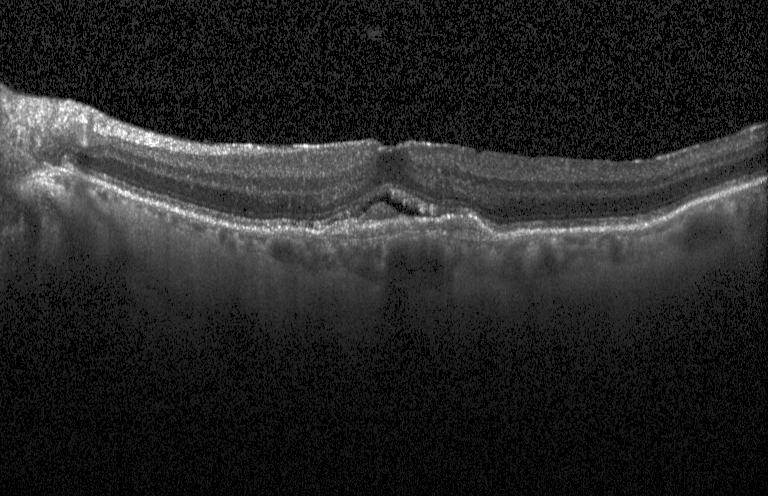
Macular OCT: choroidal neovascularization.